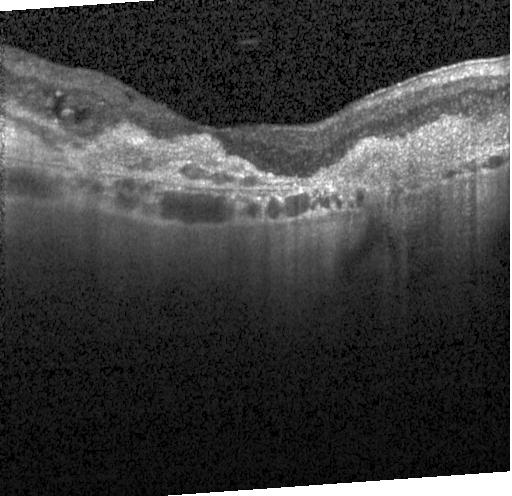

Retinal OCT B-scan
The scan shows a choroidal neovascular membrane.